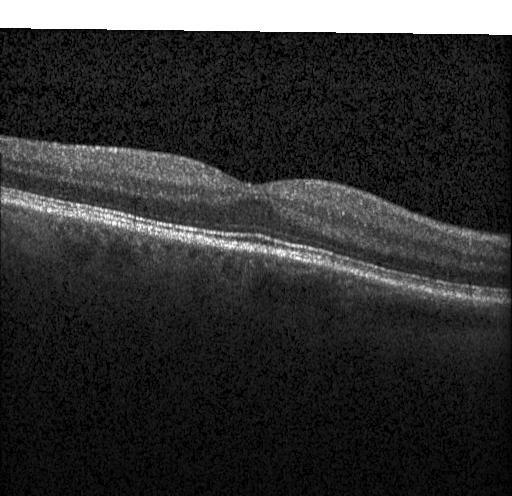 Through the macula, SD-OCT, Heidelberg Spectralis OCT system, OCT line scan.
This B-scan demonstrates no choroidal neovascularization, no diabetic macular edema, and no drusen.